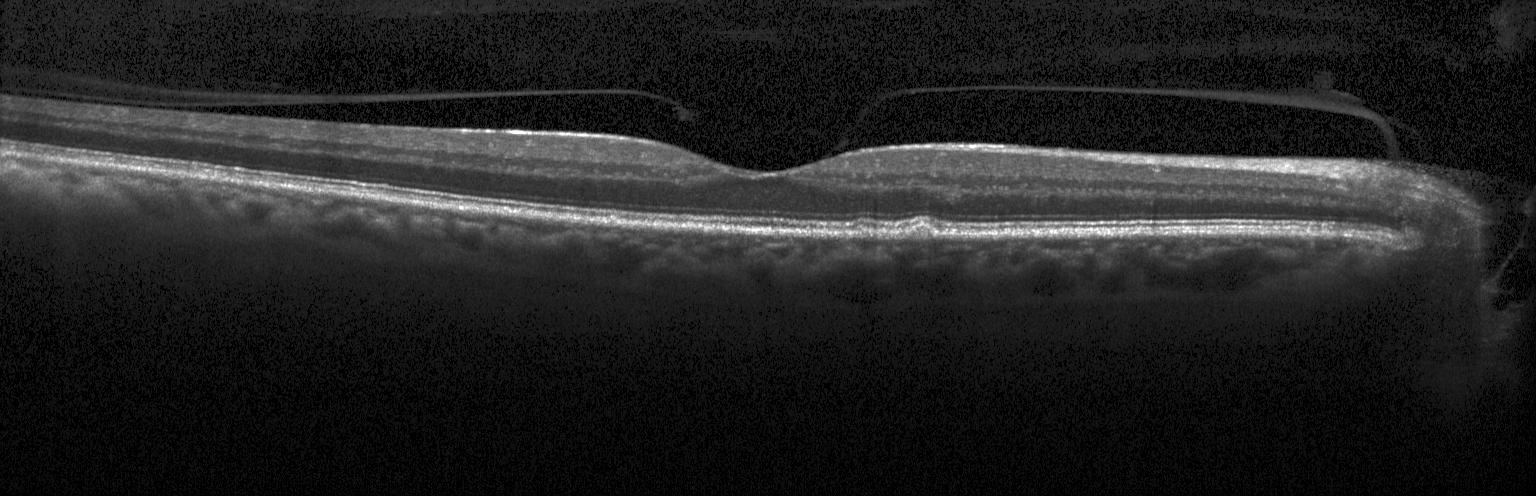
Horizontal scan through the fovea. Retinal OCT B-scan. Instrument: Heidelberg Spectralis. SD-OCT — Finding: multiple drusen.